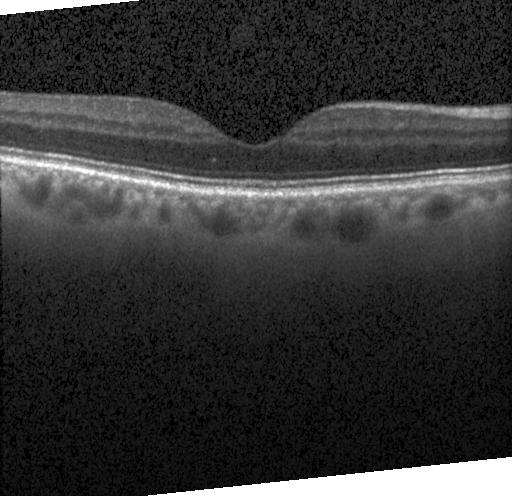

OCT line scan.
Dx: no choroidal neovascularization, no diabetic macular edema, and no drusen.